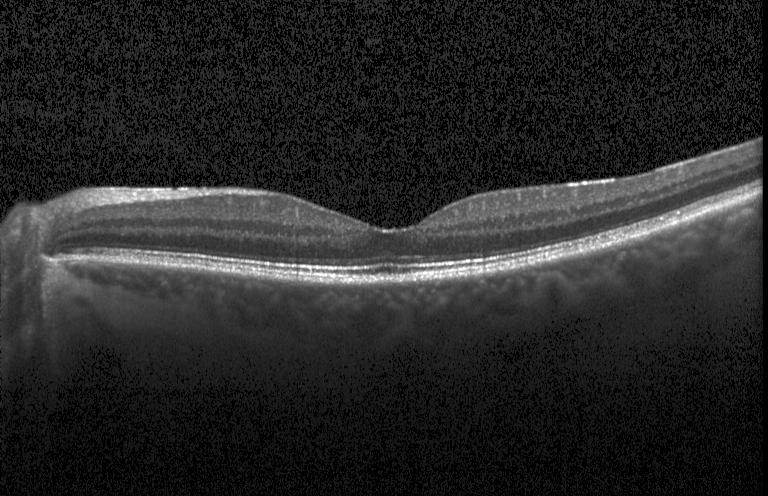 Centered on the fovea · Heidelberg Spectralis OCT system · optical coherence tomography scan.
Impression: no choroidal neovascularization, no diabetic macular edema, and no drusen.